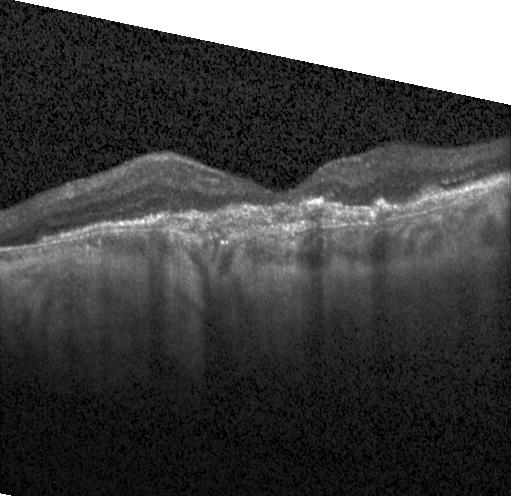 OCT B-scan showing a choroidal neovascular membrane.